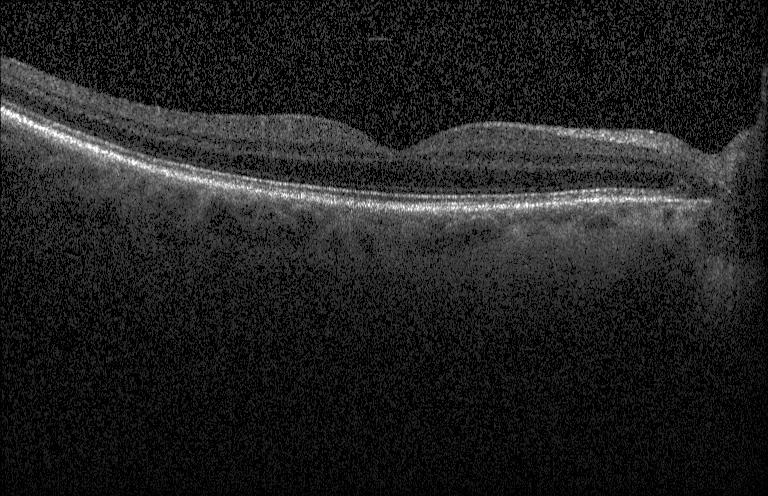

Optical coherence tomography B-scan
Diagnosis: no evidence of choroidal neovascularization, diabetic macular edema, or drusen.